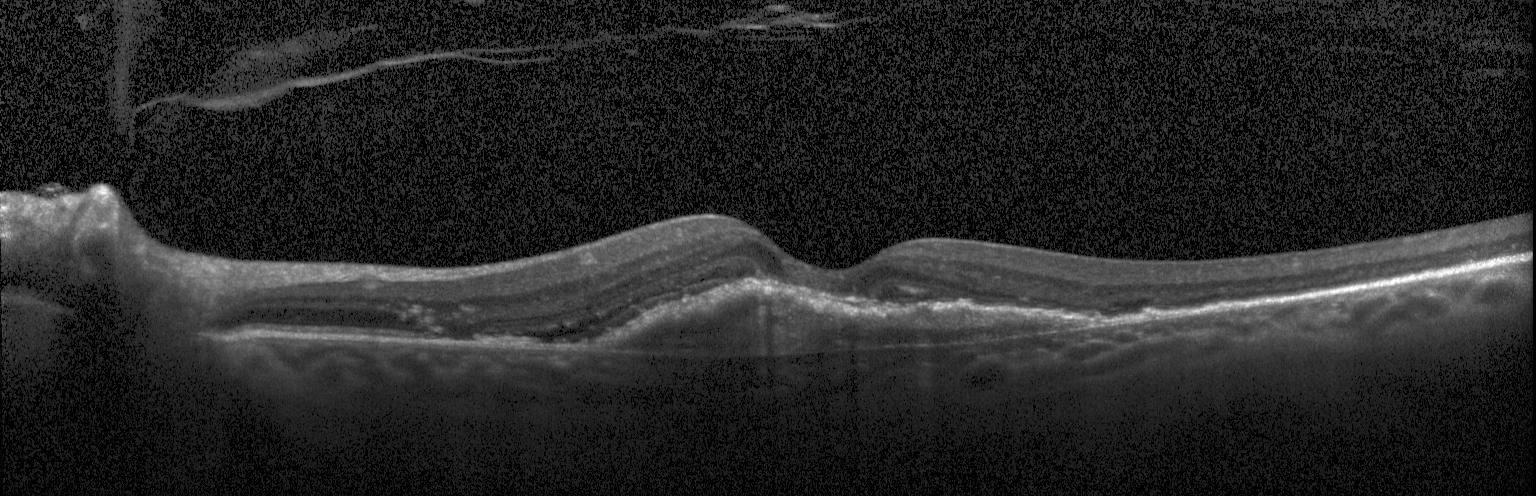
Optical coherence tomography B-scan, spectral-domain OCT, acquired on a Heidelberg Spectralis, fovea-centered. This B-scan demonstrates choroidal neovascularization (CNV).